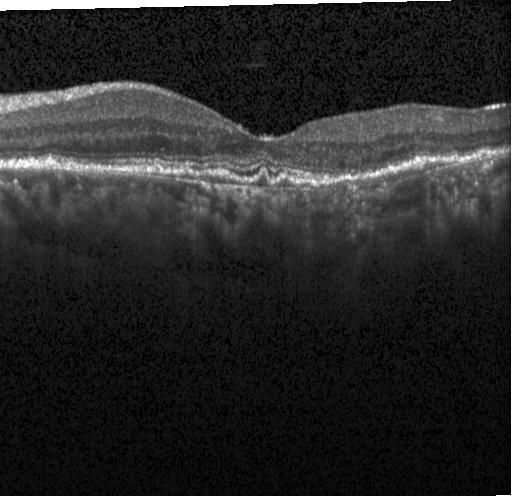
Spectral-domain optical coherence tomography, Heidelberg Spectralis OCT system, OCT line scan, fovea-centered — Diagnosis: a choroidal neovascular membrane.